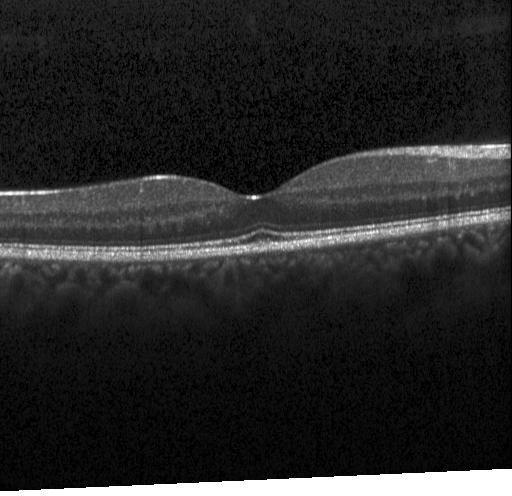

Through the macula · spectral-domain optical coherence tomography · instrument: Heidelberg Spectralis · OCT B-scan — Macular OCT: no evidence of choroidal neovascularization, diabetic macular edema, or drusen.